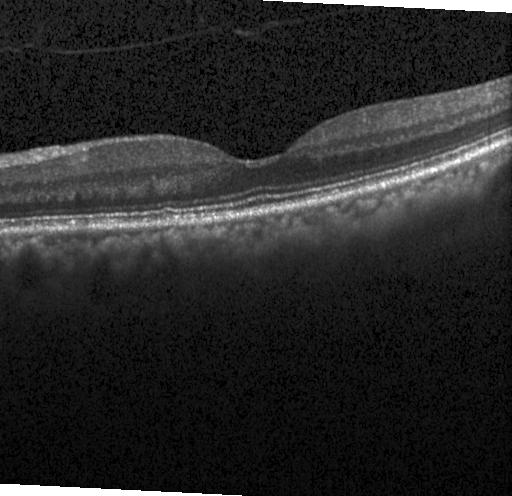
Retinal OCT B-scan. Spectral-domain OCT. Acquired on a Heidelberg Spectralis. Macular scan. OCT finding: no choroidal neovascularization, no diabetic macular edema, and no drusen.